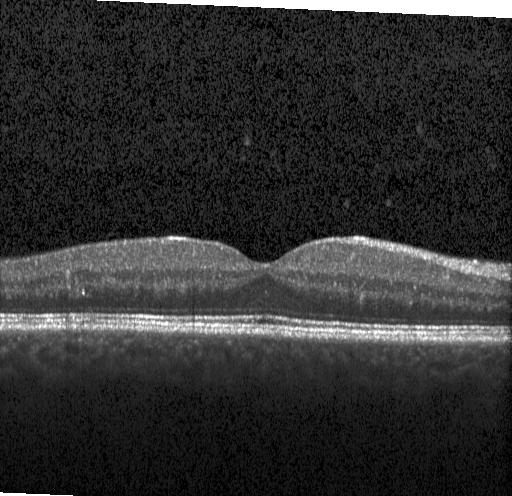 Macular OCT demonstrating no CNV, no DME, and no drusen.